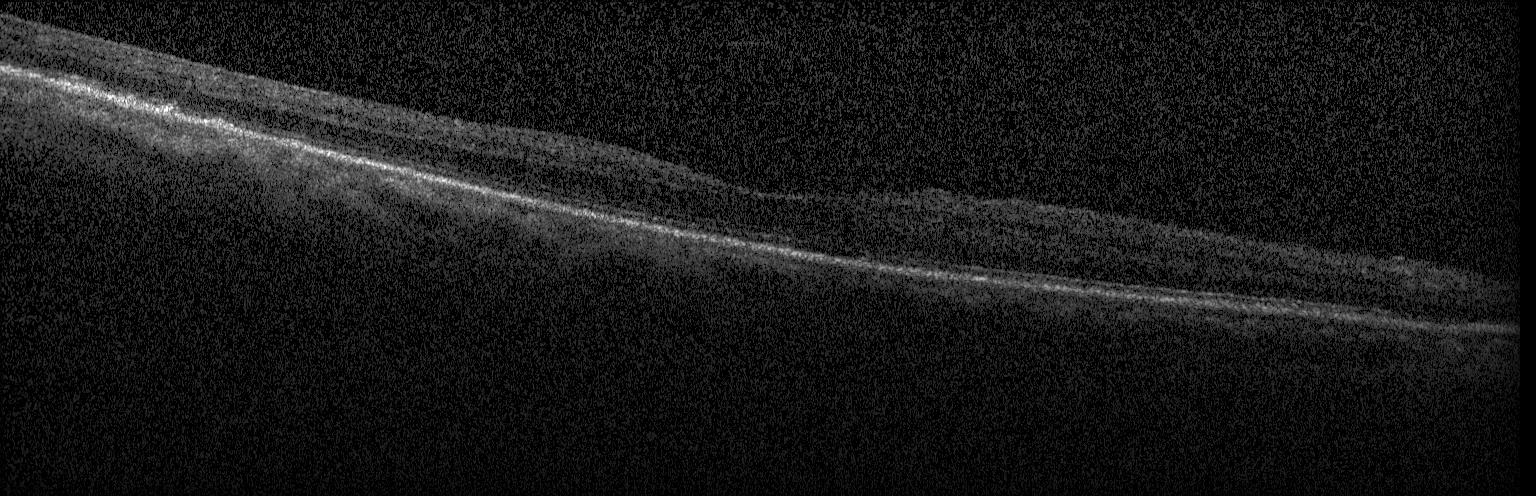
OCT finding: neither choroidal neovascularization, diabetic macular edema, nor drusen.